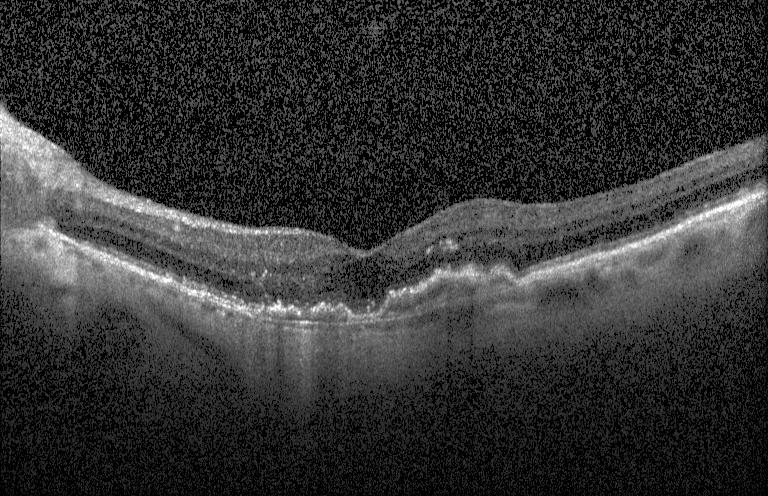
OCT scan showing CNV.